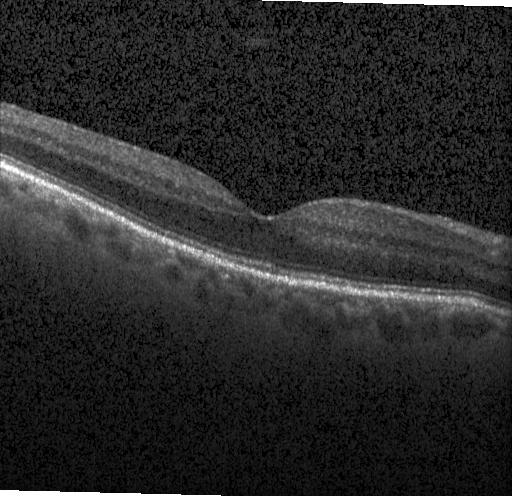

Finding: no evidence of choroidal neovascularization, diabetic macular edema, or drusen.